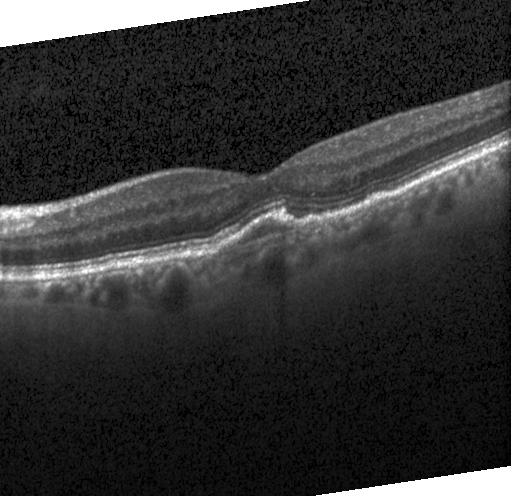

Spectral-domain OCT, optical coherence tomography B-scan, instrument: Heidelberg Spectralis
Impression: choroidal neovascularization.